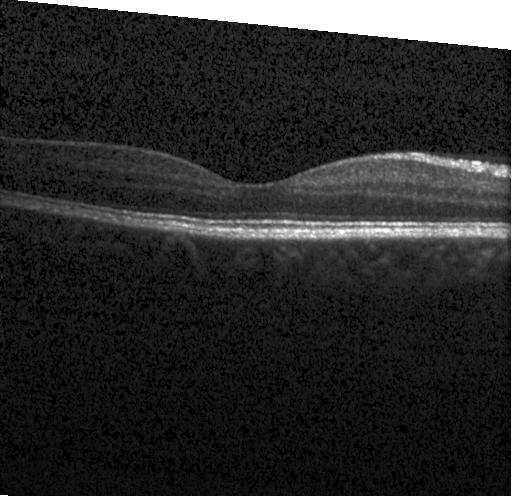
Fovea-centered; spectral-domain OCT; retinal OCT cross-section; acquired on a Heidelberg Spectralis. Finding: neither choroidal neovascularization, diabetic macular edema, nor drusen.